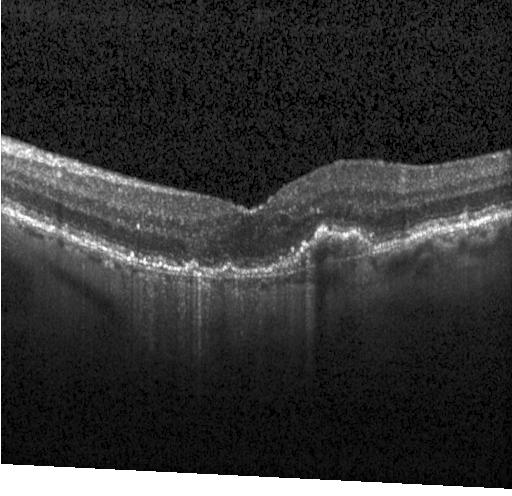
OCT B-scan
Impression: a choroidal neovascular membrane.